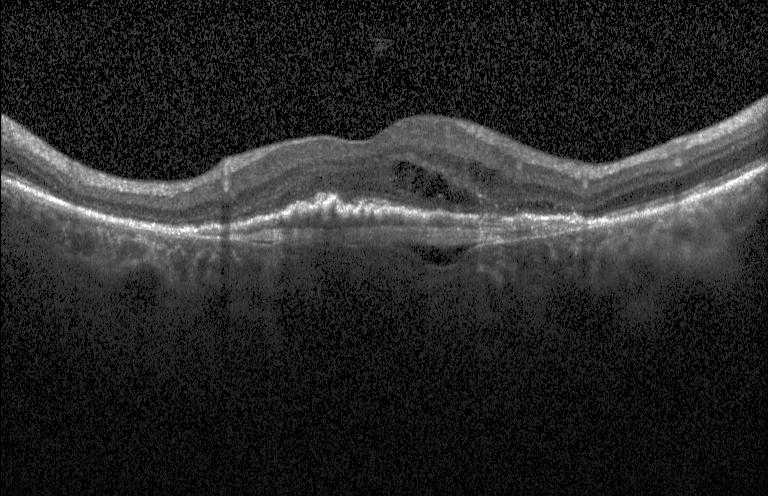

OCT line scan · SD-OCT
Choroidal neovascularization.